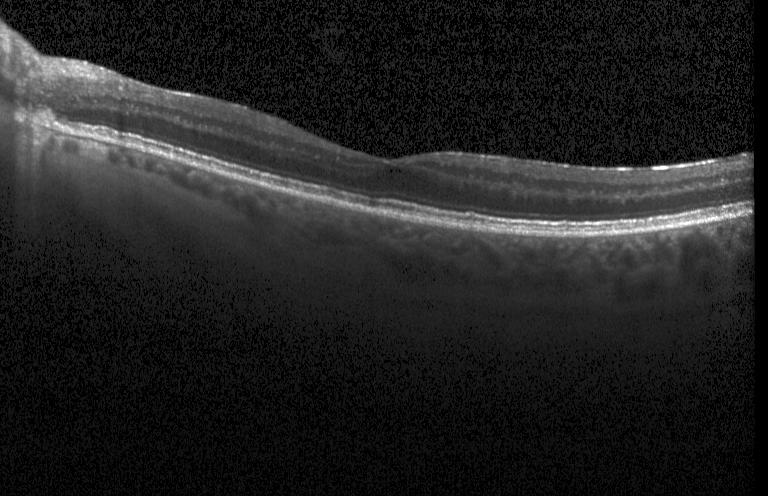 Retinal OCT cross-section; SD-OCT.
Impression: no choroidal neovascularization, no diabetic macular edema, and no drusen.